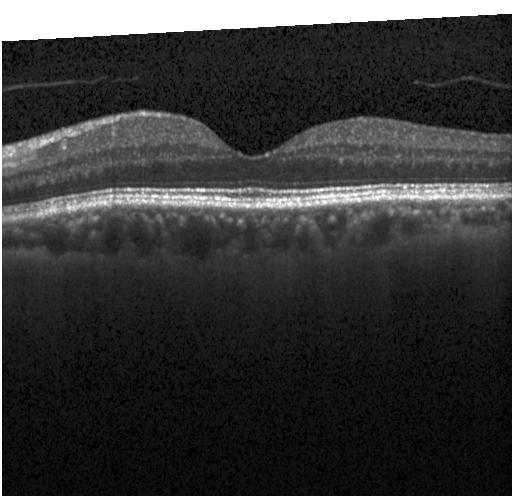 Assessment: neither CNV, DME, nor drusen.